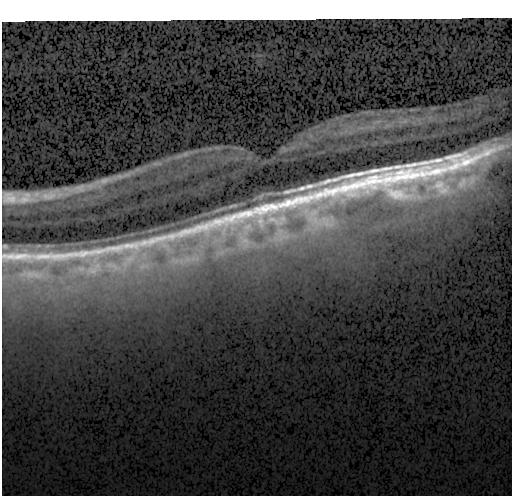

Diagnosis: no CNV, no DME, and no drusen.